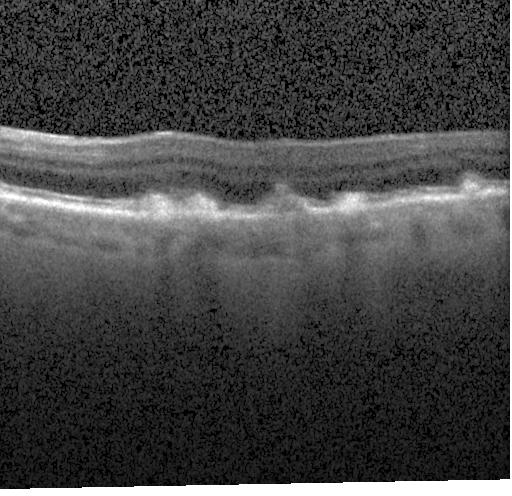
Retinal OCT cross-section; horizontal scan through the fovea; spectral-domain optical coherence tomography; instrument: Heidelberg Spectralis. The scan shows multiple drusen.